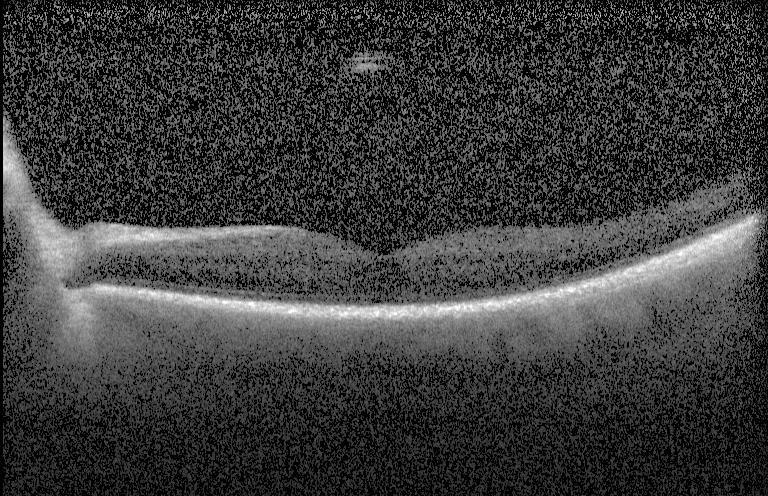

OCT scan showing no choroidal neovascularization, no diabetic macular edema, and no drusen.